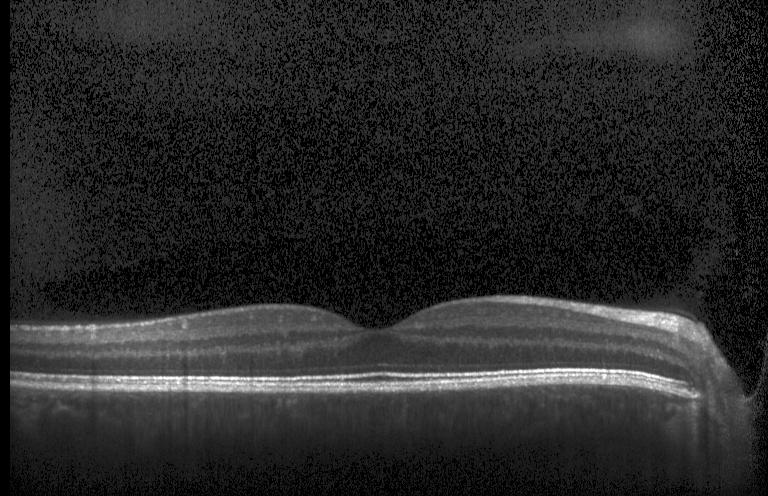 Instrument: Heidelberg Spectralis. Optical coherence tomography B-scan. SD-OCT. Macular scan
Assessment: neither choroidal neovascularization, diabetic macular edema, nor drusen.